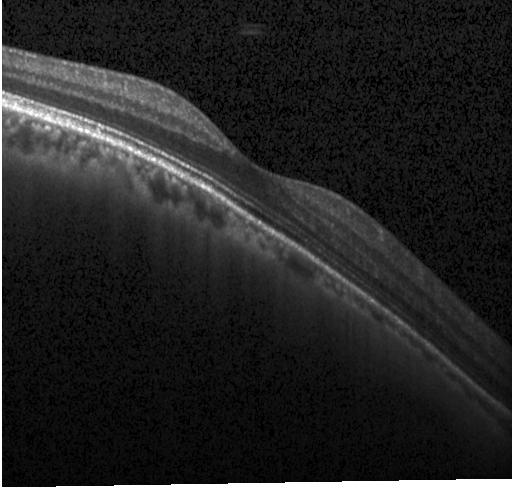

Optical coherence tomography scan, spectral-domain optical coherence tomography — Finding: no evidence of choroidal neovascularization, diabetic macular edema, or drusen.